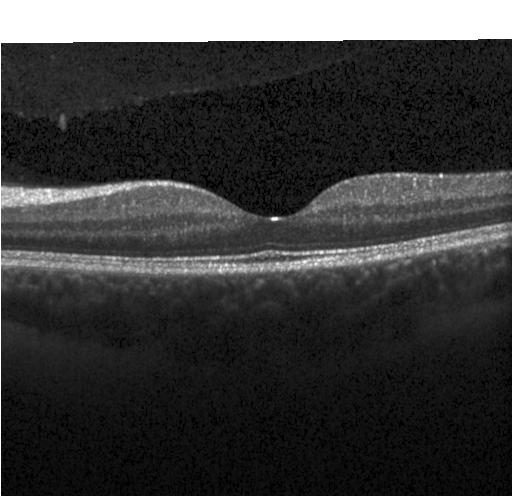
OCT line scan
Impression: no choroidal neovascularization, no diabetic macular edema, and no drusen.